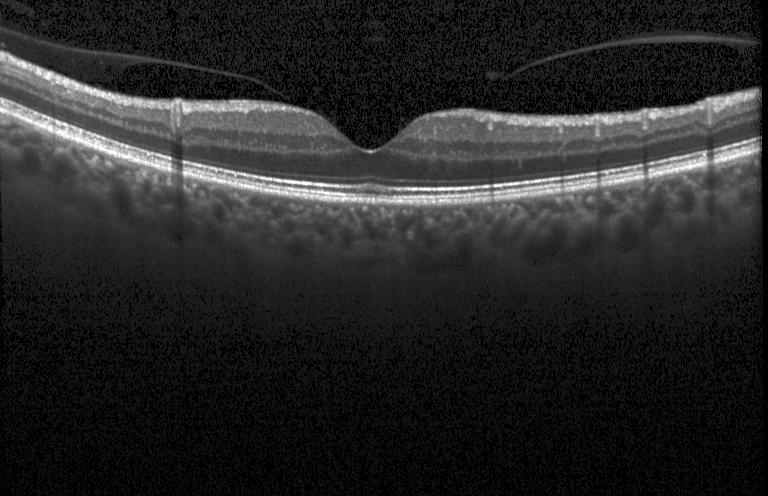 Heidelberg Spectralis OCT system · OCT B-scan · spectral-domain OCT · centered on the fovea. The scan shows neither choroidal neovascularization, diabetic macular edema, nor drusen.